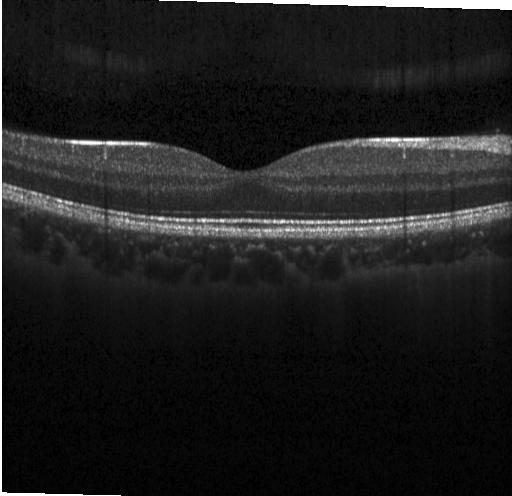
Heidelberg Spectralis OCT system, optical coherence tomography scan, spectral-domain optical coherence tomography, horizontal scan through the fovea.
Assessment: no choroidal neovascularization, diabetic macular edema, or drusen.